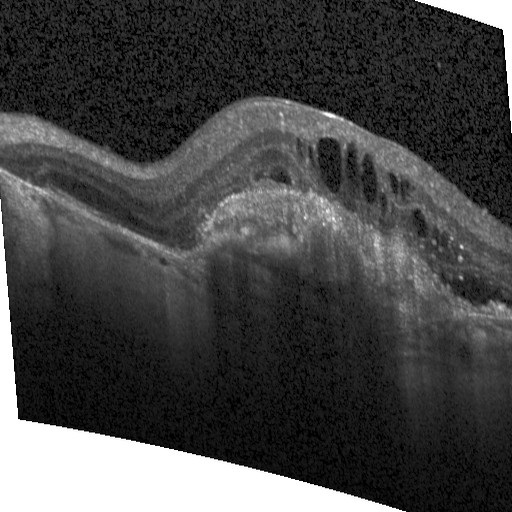 Macular OCT demonstrating diabetic macular edema.